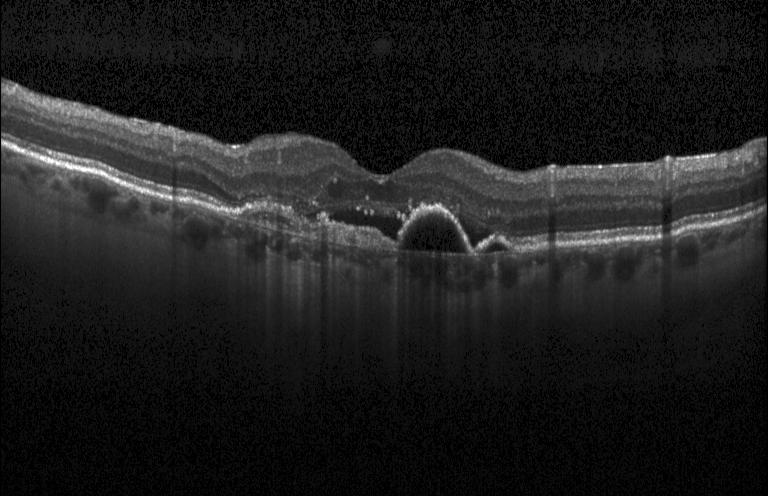 OCT B-scan — Dx: a choroidal neovascular membrane.